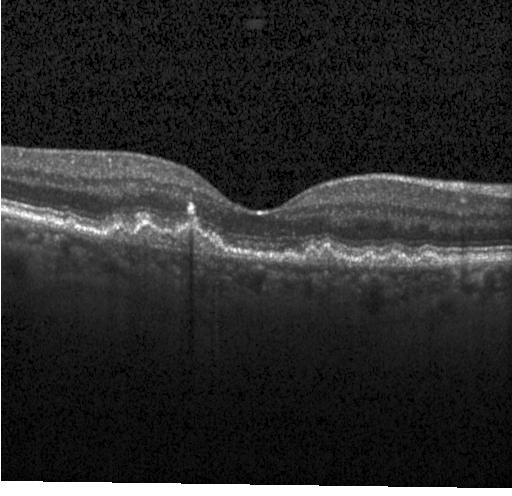
OCT B-scan.
Finding: CNV.